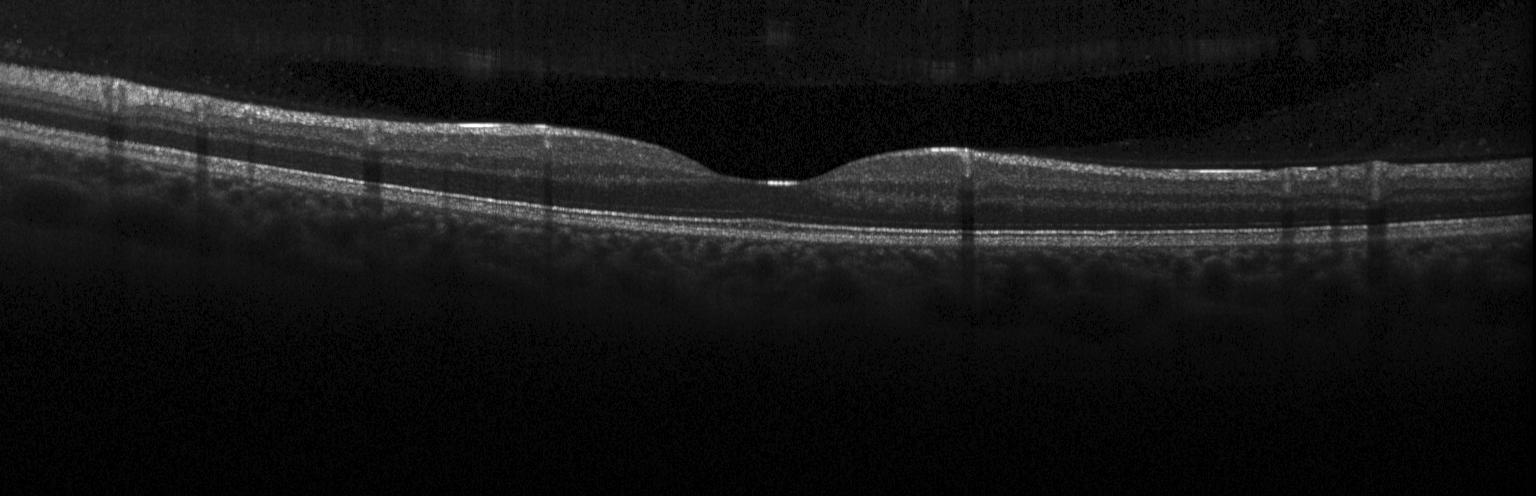 Heidelberg Spectralis OCT system; SD-OCT; optical coherence tomography scan; centered on the fovea
The scan shows no choroidal neovascularization, diabetic macular edema, or drusen.